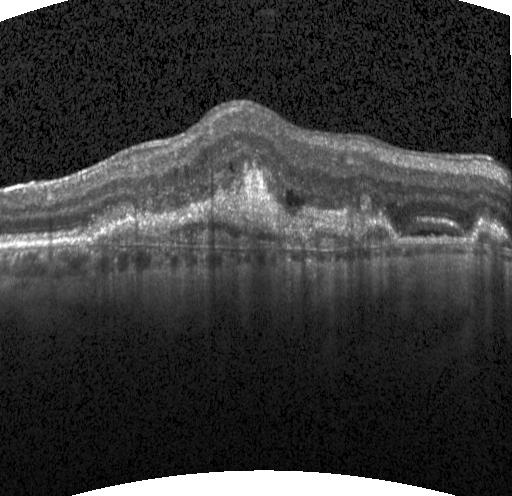
Through the macula; retinal OCT B-scan; Heidelberg Spectralis. Dx: choroidal neovascularization (CNV).